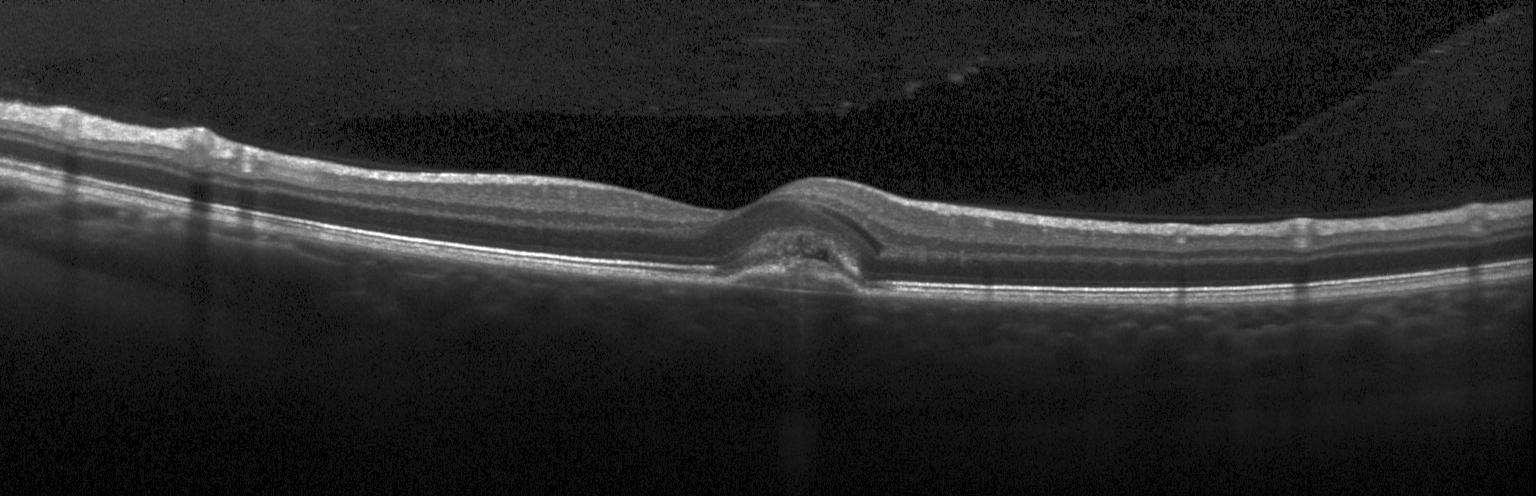 This B-scan demonstrates a choroidal neovascular membrane.